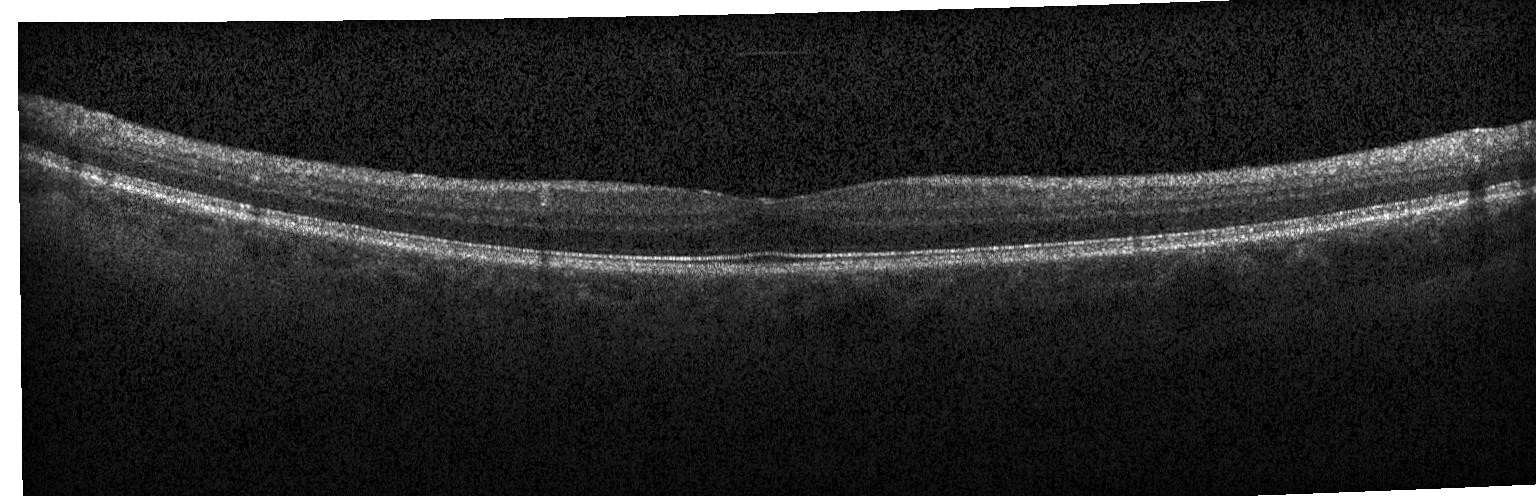
Impression: no choroidal neovascularization, diabetic macular edema, or drusen.